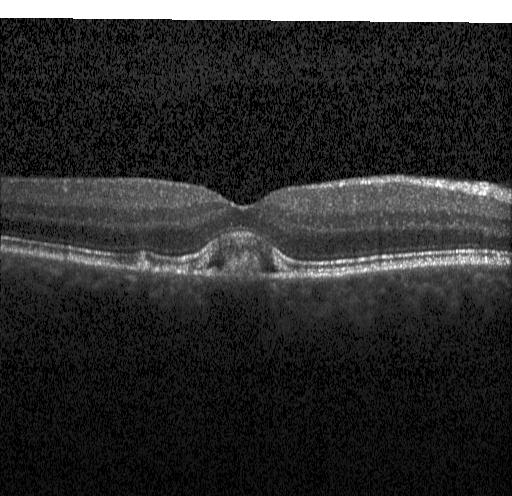 OCT B-scan · Heidelberg Spectralis · spectral-domain optical coherence tomography.
The scan shows a choroidal neovascular membrane.